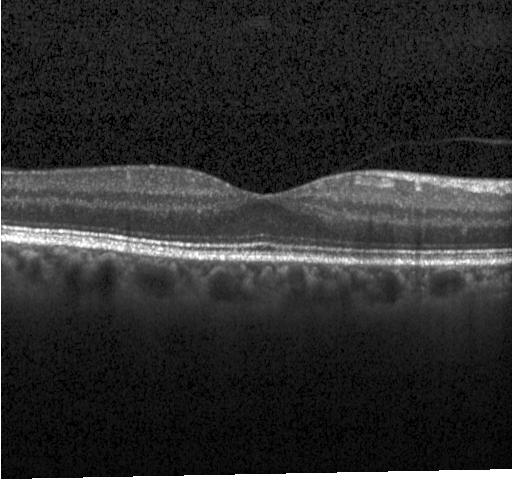
OCT B-scan. Heidelberg Spectralis. Macular scan. Spectral-domain optical coherence tomography.
Finding: no CNV, DME, or drusen.